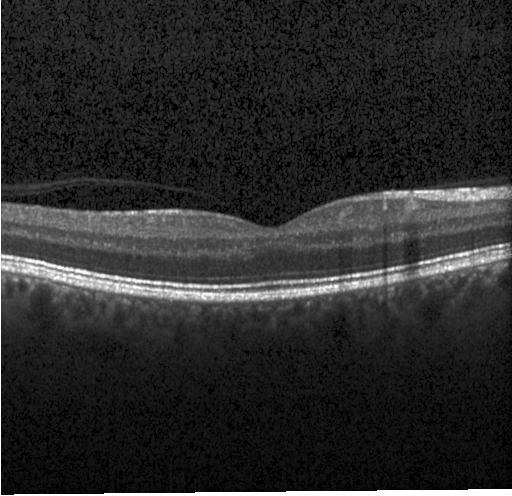

OCT B-scan. This B-scan demonstrates neither choroidal neovascularization, diabetic macular edema, nor drusen.